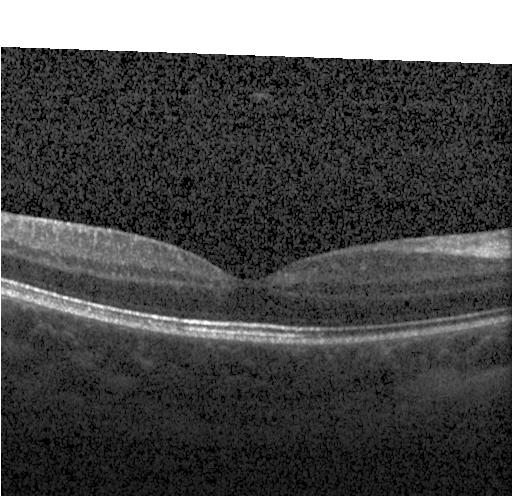
Macular OCT demonstrating no choroidal neovascularization, diabetic macular edema, or drusen.